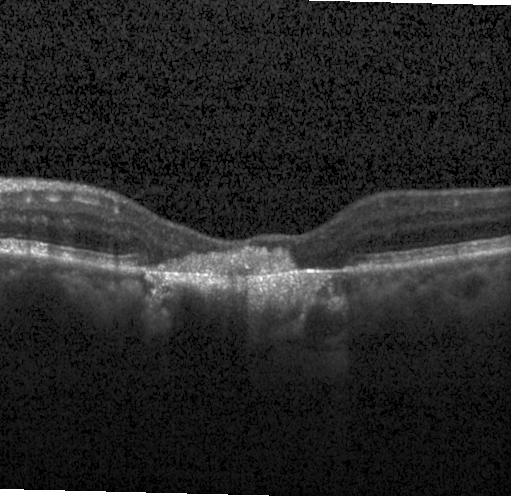
OCT B-scan — Impression: a choroidal neovascular membrane.